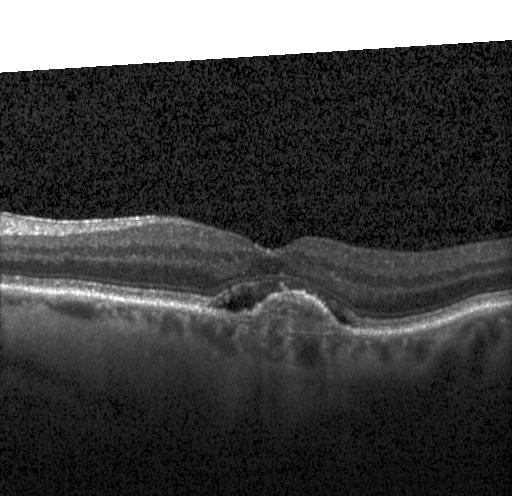 Finding: CNV.